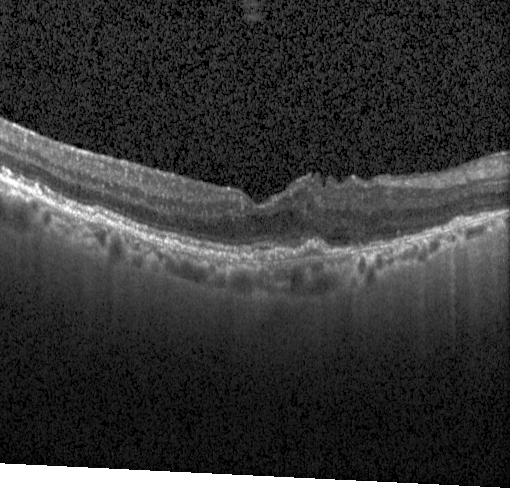

Optical coherence tomography B-scan — Assessment: a choroidal neovascular membrane.